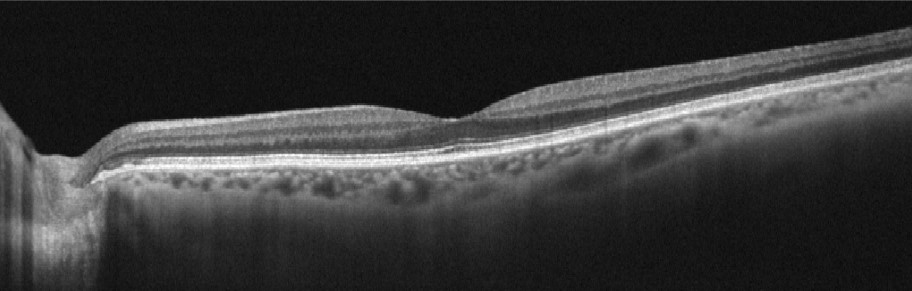
Retinal OCT B-scan. Fovea-centered. Acquired on an Optovue Avanti RTVue XR. This B-scan demonstrates no evidence of AMD, DME, ERM, RAO, RVO, or VID.